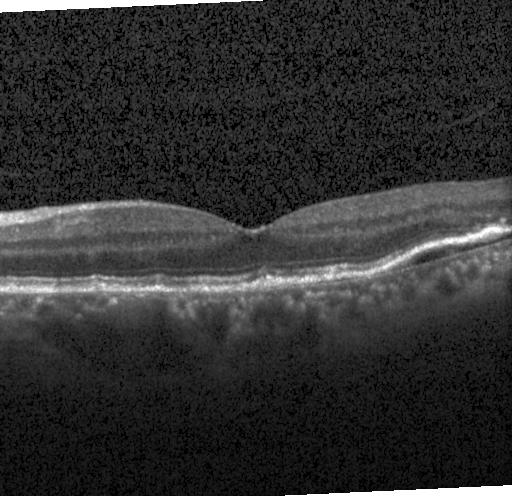
Through the macula. OCT line scan. Instrument: Heidelberg Spectralis.
A choroidal neovascular membrane.